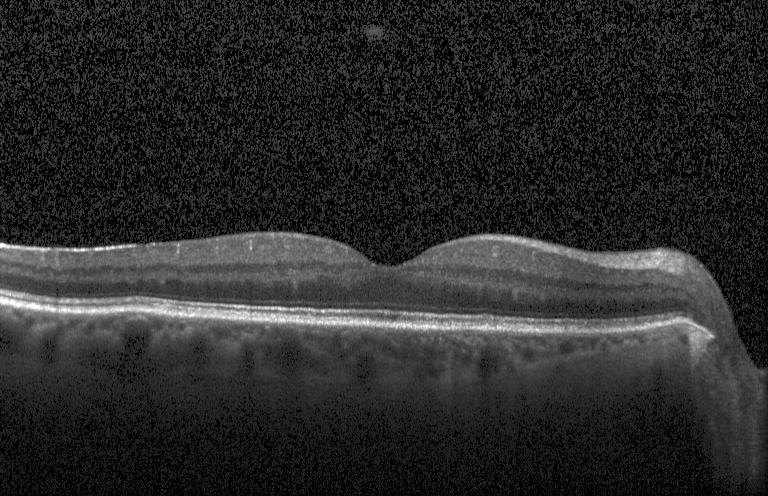

Spectral-domain OCT B-scan: no evidence of CNV, DME, or drusen.